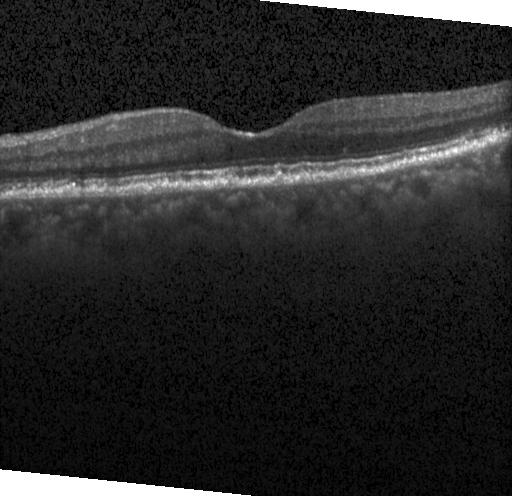

OCT B-scan — Finding: sub-RPE drusenoid deposits.